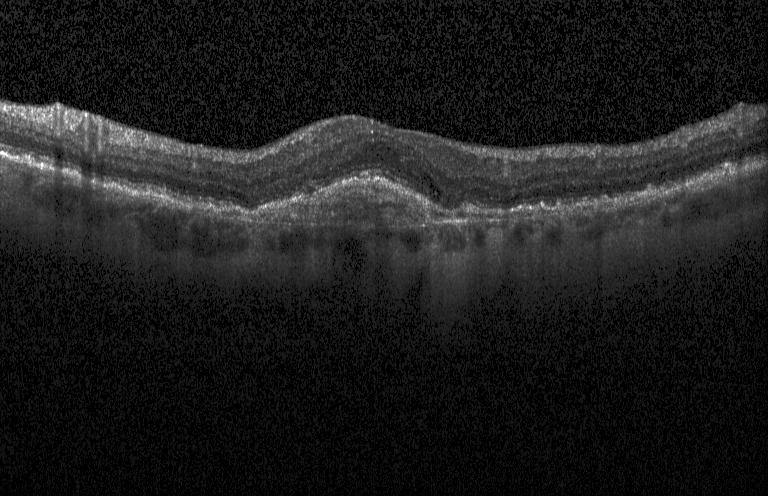 SD-OCT; horizontal scan through the fovea; acquired on a Heidelberg Spectralis; retinal OCT cross-section — A choroidal neovascular membrane.